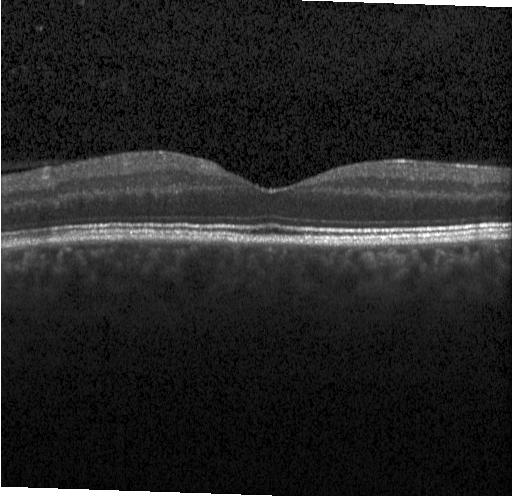

Macular OCT: no evidence of CNV, DME, or drusen.